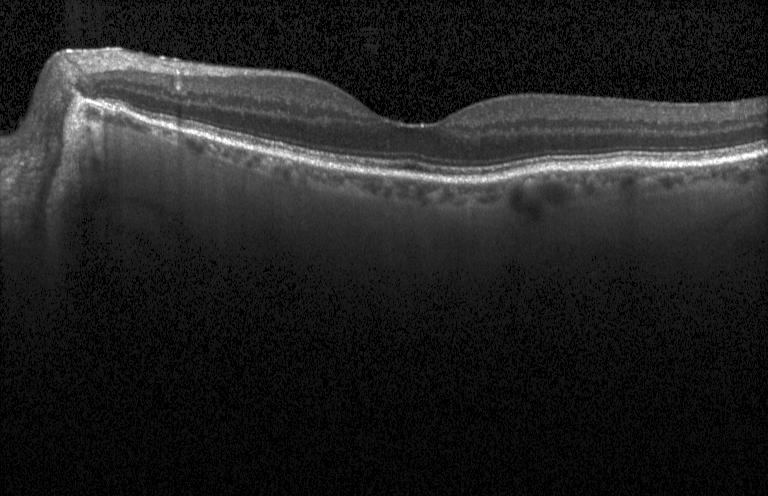

Retinal OCT B-scan — The scan shows no choroidal neovascularization, no diabetic macular edema, and no drusen.